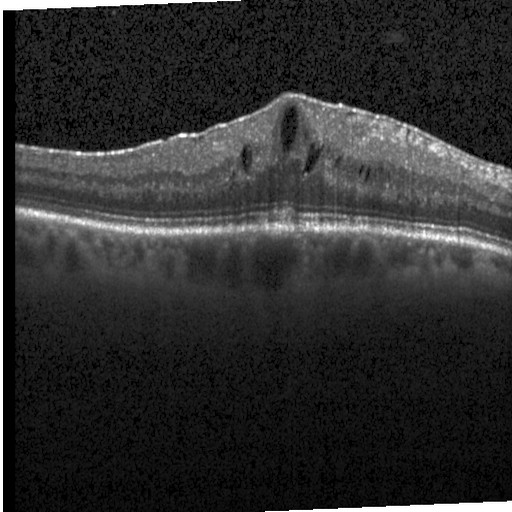

Retinal OCT cross-section, macular scan — Diagnosis: diabetic macular edema.